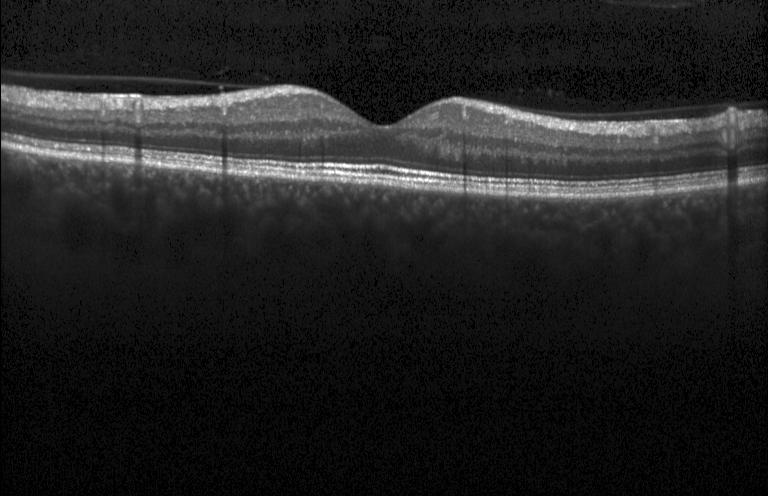

Macular OCT demonstrating neither CNV, DME, nor drusen.